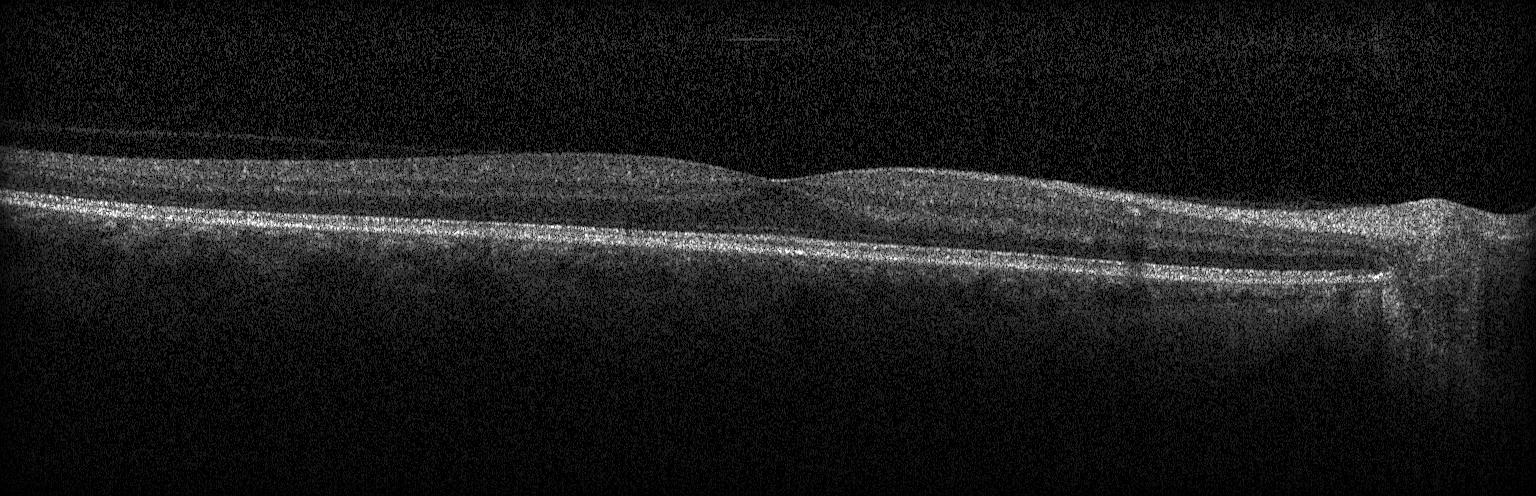 SD-OCT. Heidelberg Spectralis. Fovea-centered. OCT line scan. This B-scan demonstrates neither choroidal neovascularization, diabetic macular edema, nor drusen.